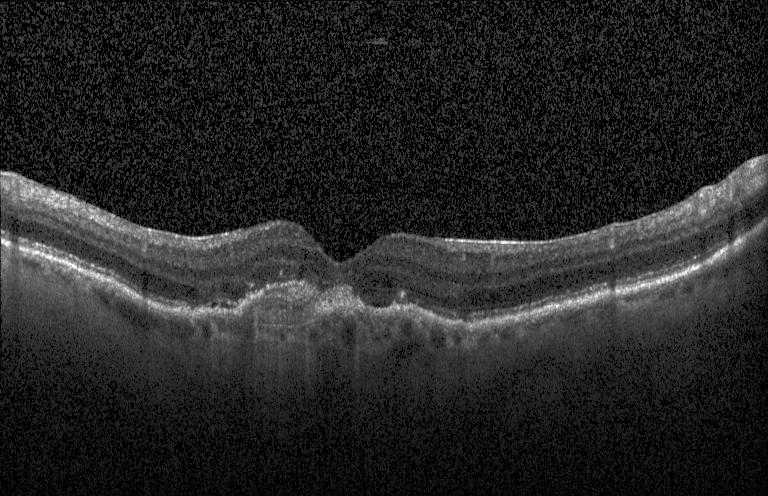 Spectral-domain optical coherence tomography. Instrument: Heidelberg Spectralis. Fovea-centered. Retinal OCT cross-section. Assessment: a choroidal neovascular membrane.